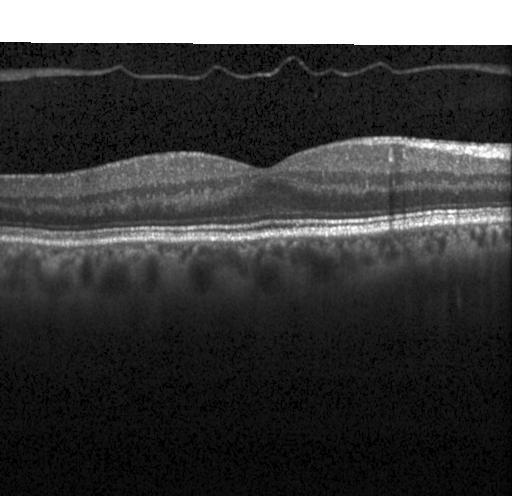

Finding: no choroidal neovascularization, no diabetic macular edema, and no drusen.